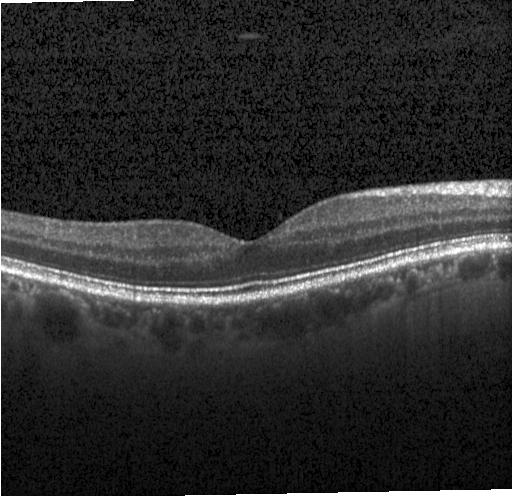
SD-OCT, acquired on a Heidelberg Spectralis, OCT B-scan
Impression: no choroidal neovascularization, no diabetic macular edema, and no drusen.